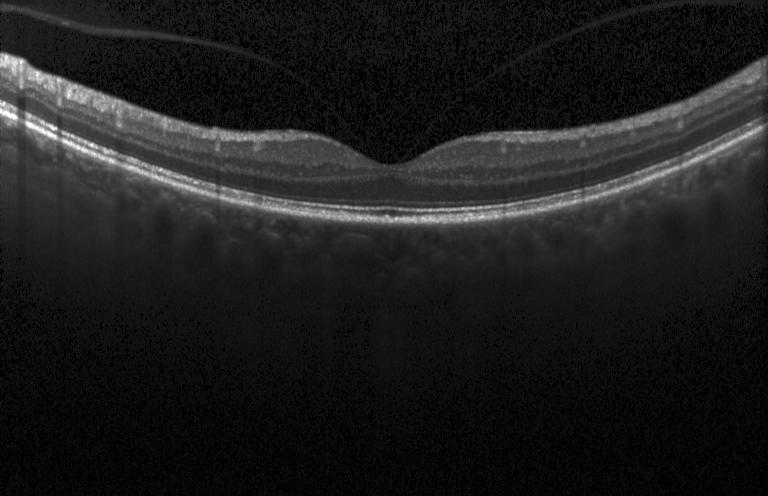
OCT line scan. Acquired on a Heidelberg Spectralis. Horizontal scan through the fovea. SD-OCT
Assessment: neither choroidal neovascularization, diabetic macular edema, nor drusen.